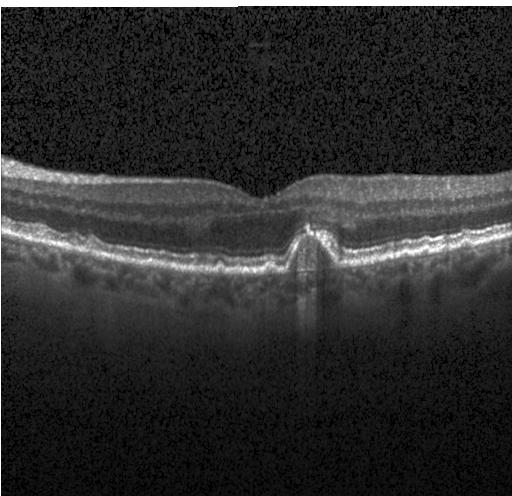 SD-OCT, Heidelberg Spectralis OCT system, optical coherence tomography B-scan
Drusen.